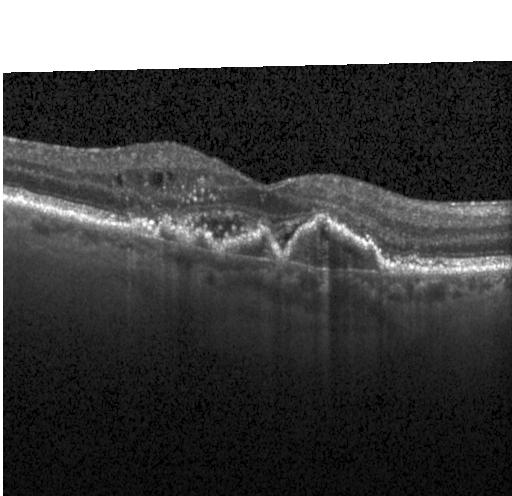
Retinal OCT cross-section, spectral-domain optical coherence tomography, instrument: Heidelberg Spectralis. Diagnosis: choroidal neovascularization (CNV).